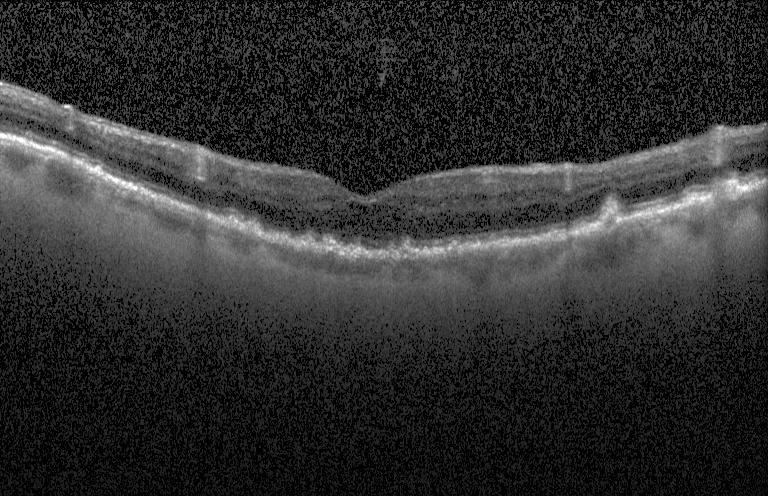 Impression: a choroidal neovascular membrane.